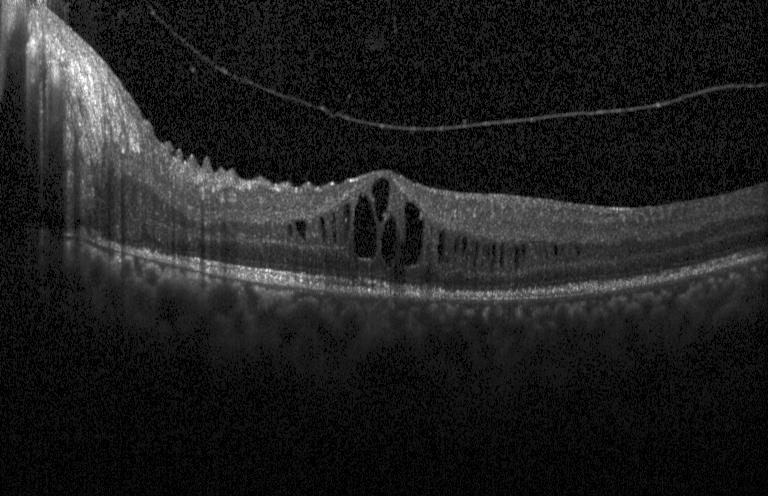 Macular OCT demonstrating DME.